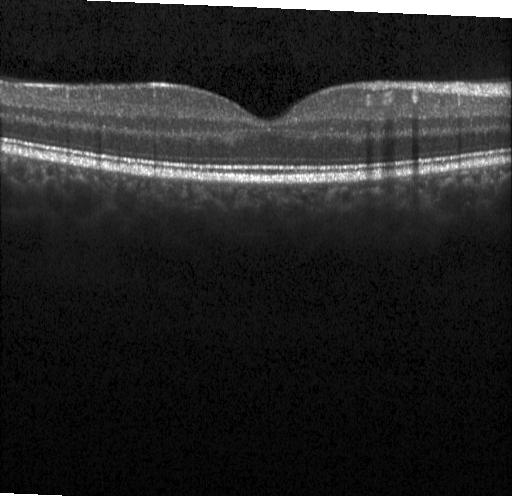
Impression: neither choroidal neovascularization, diabetic macular edema, nor drusen.